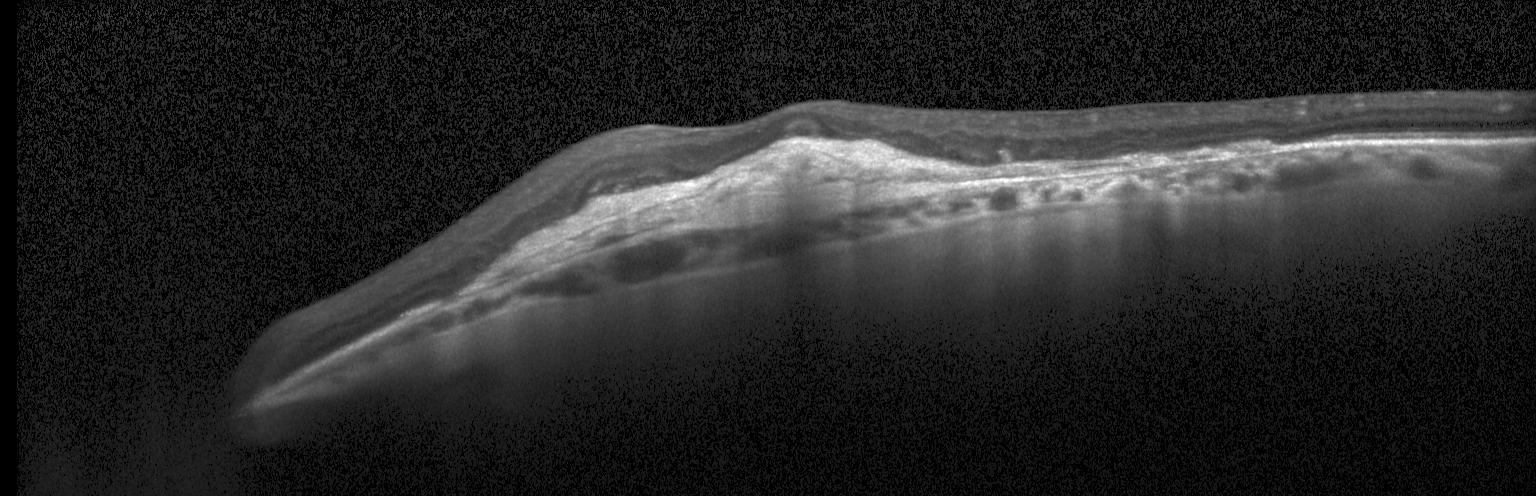
Retinal OCT B-scan. Diagnosis: choroidal neovascularization.